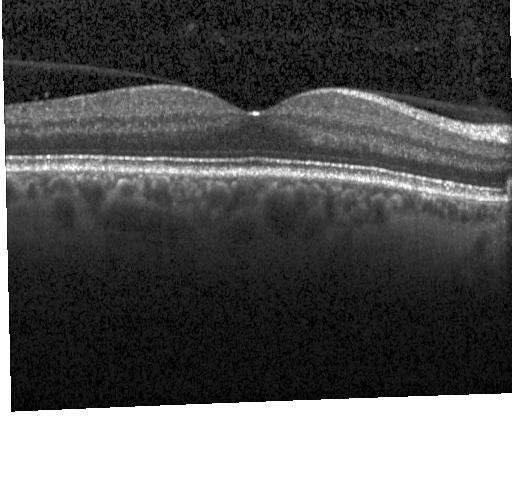
The scan shows no CNV, no DME, and no drusen.